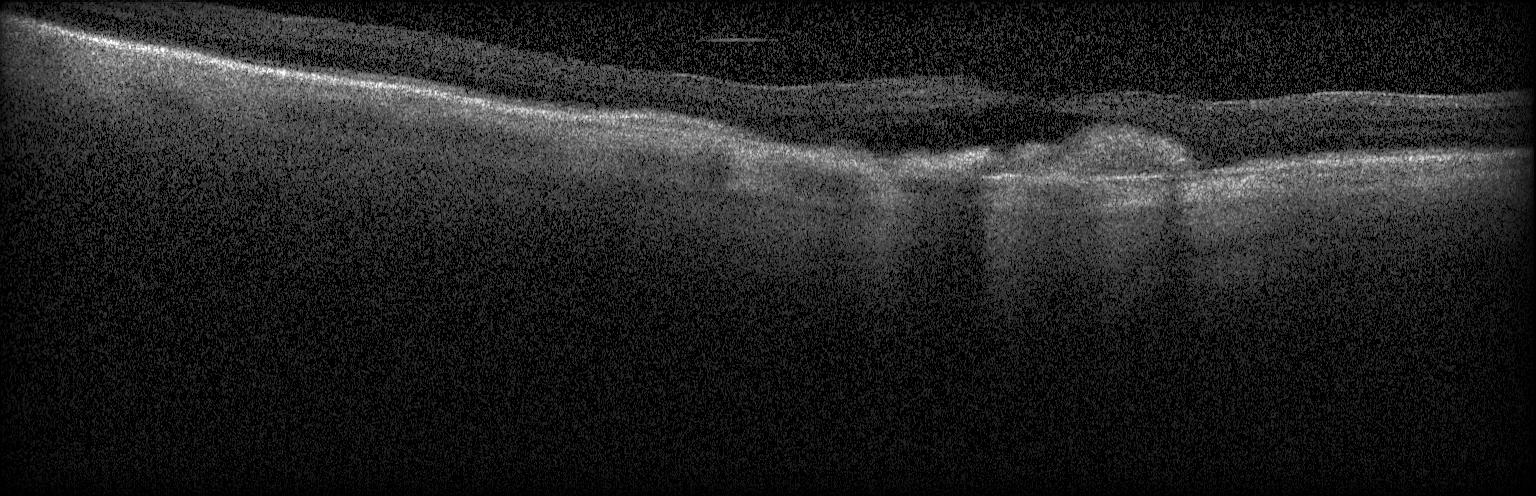
Dx: choroidal neovascularization (CNV).